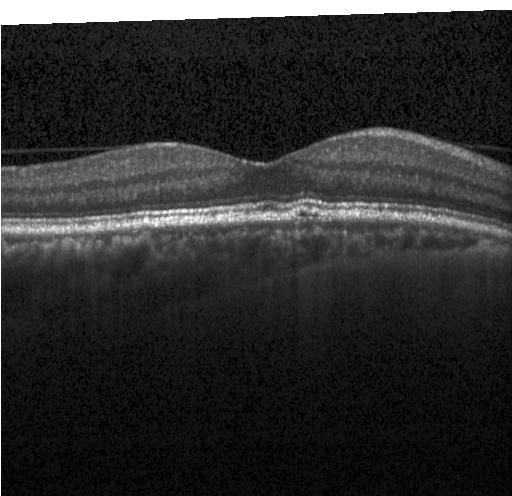

OCT line scan
This B-scan demonstrates drusen.